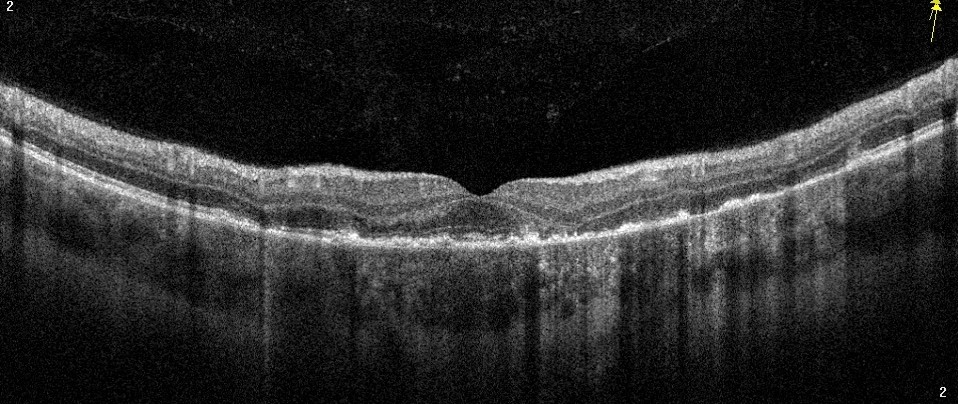 Assessment: age-related macular degeneration.